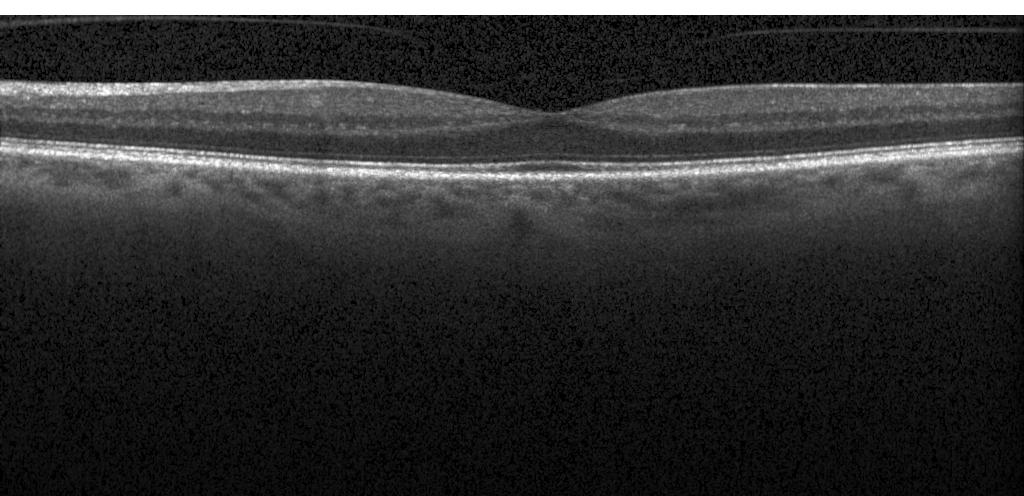
Impression: no choroidal neovascularization, diabetic macular edema, or drusen.